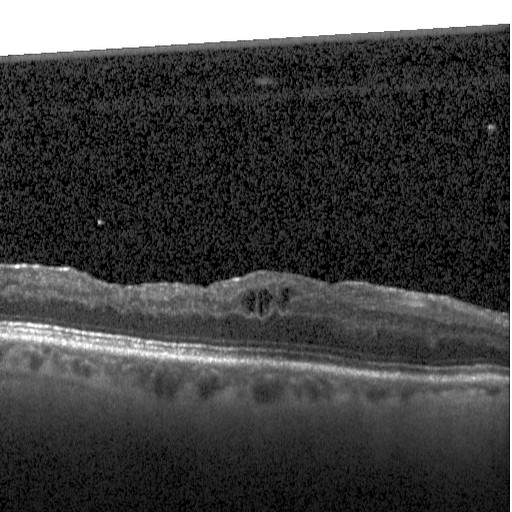 Retinal OCT B-scan.
The scan shows DME.